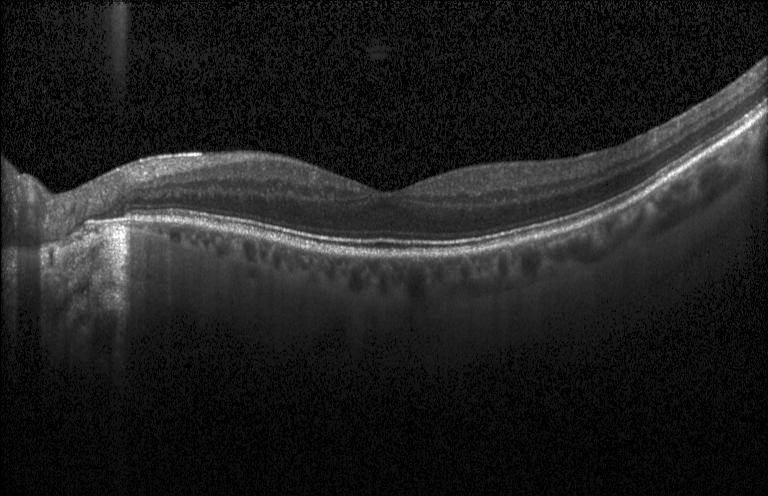

Retinal OCT B-scan — OCT finding: no CNV, DME, or drusen.